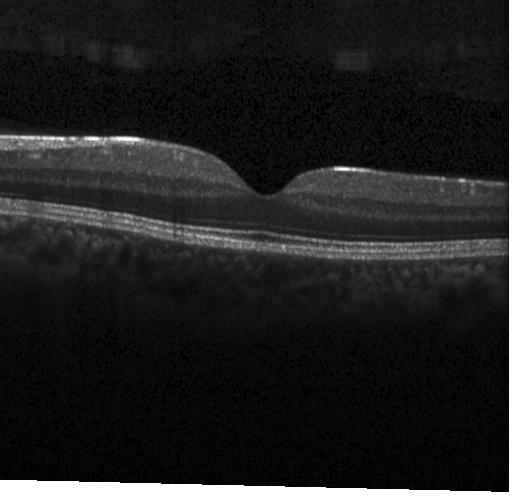

OCT finding: no CNV, DME, or drusen.